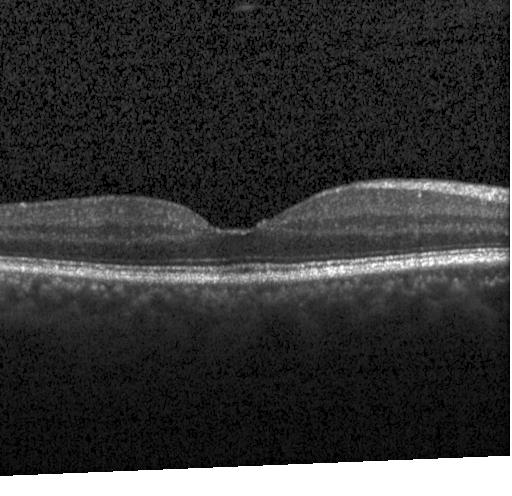
Diagnosis: no evidence of CNV, DME, or drusen.